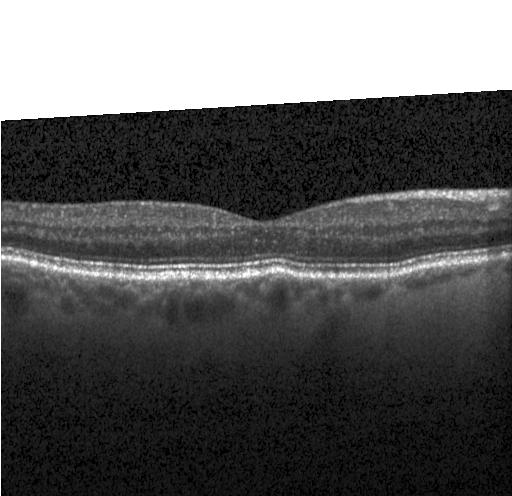
Macular OCT demonstrating no choroidal neovascularization, diabetic macular edema, or drusen.